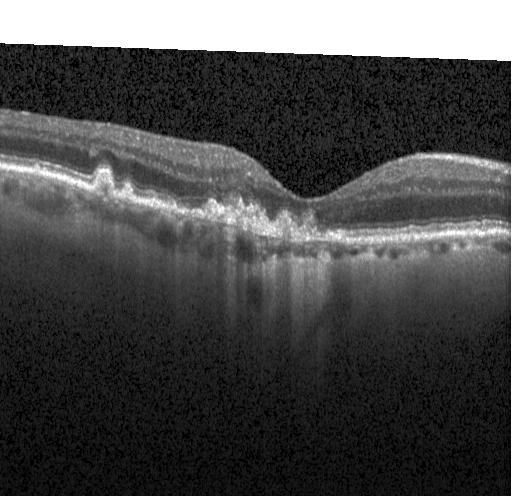 OCT line scan. SD-OCT. Macular scan.
OCT finding: choroidal neovascularization (CNV).